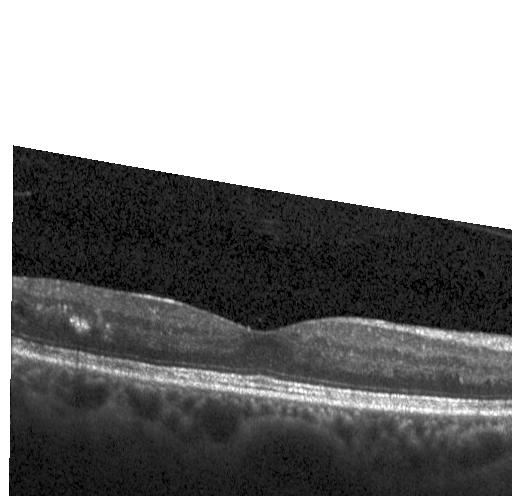 OCT B-scan; centered on the fovea; Heidelberg Spectralis
Finding: diabetic macular edema (DME).